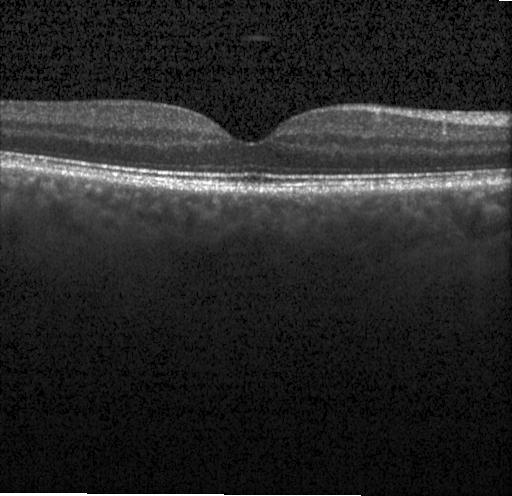
Finding: no evidence of choroidal neovascularization, diabetic macular edema, or drusen.